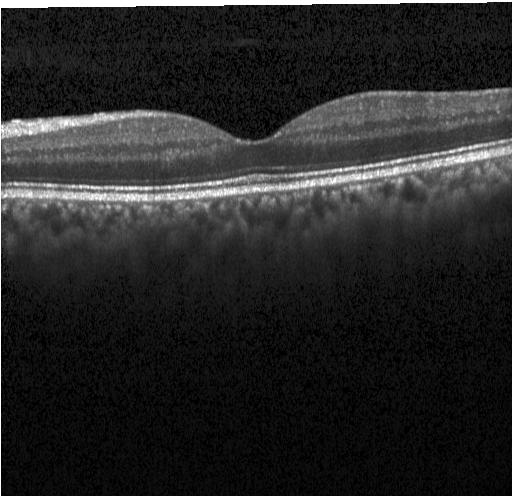 OCT line scan. Spectral-domain OCT.
No choroidal neovascularization, diabetic macular edema, or drusen.